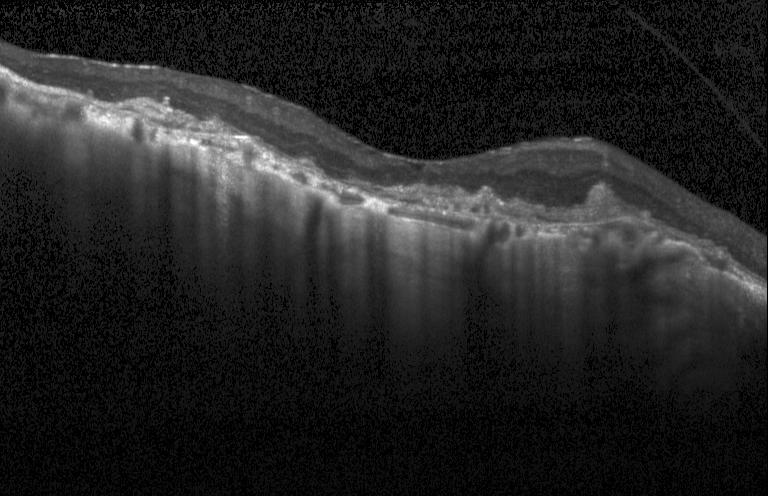 This B-scan demonstrates a choroidal neovascular membrane.